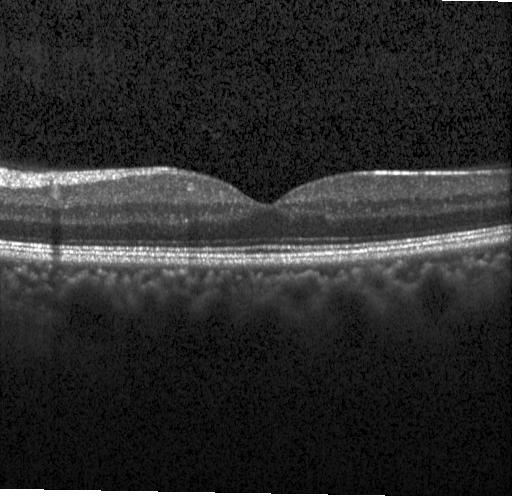

Diagnosis: no evidence of CNV, DME, or drusen.